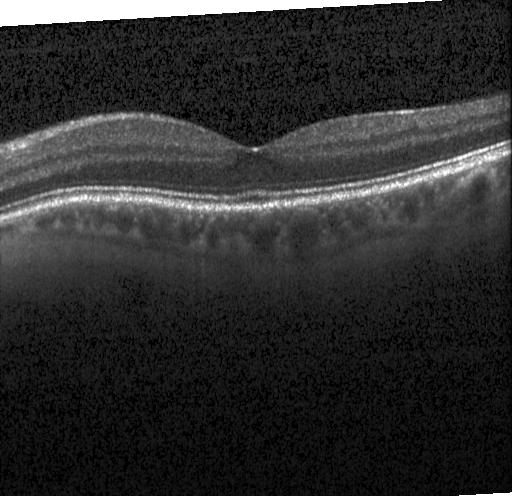 Retinal OCT B-scan. Dx: no choroidal neovascularization, diabetic macular edema, or drusen.